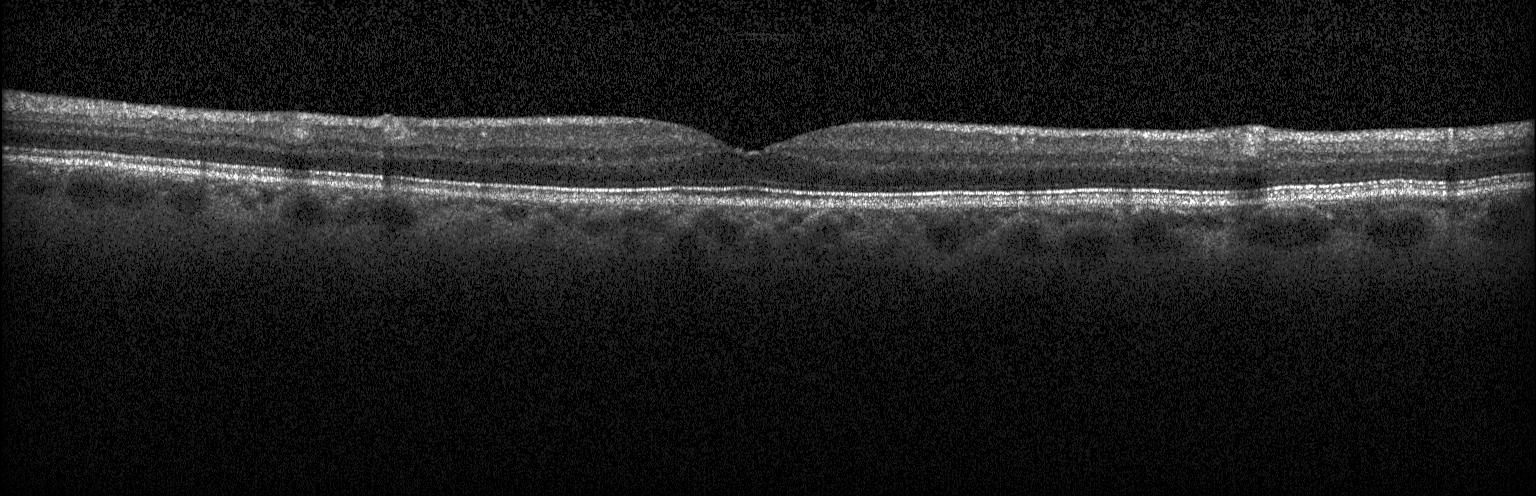

Instrument: Heidelberg Spectralis. OCT line scan. Spectral-domain OCT.
Finding: neither choroidal neovascularization, diabetic macular edema, nor drusen.